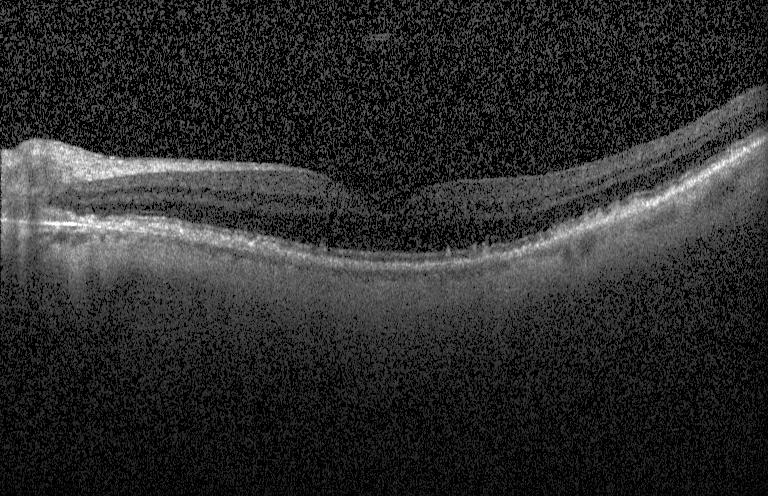

Retinal OCT B-scan. Heidelberg Spectralis OCT system. SD-OCT.
Impression: drusen.